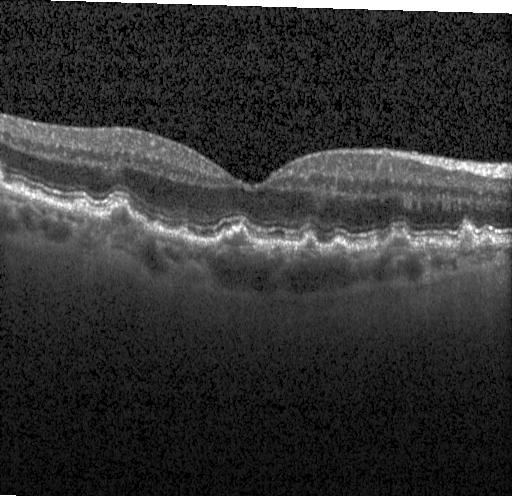
Spectral-domain OCT. Retinal OCT B-scan. Centered on the fovea. Instrument: Heidelberg Spectralis
Macular OCT: multiple drusen.